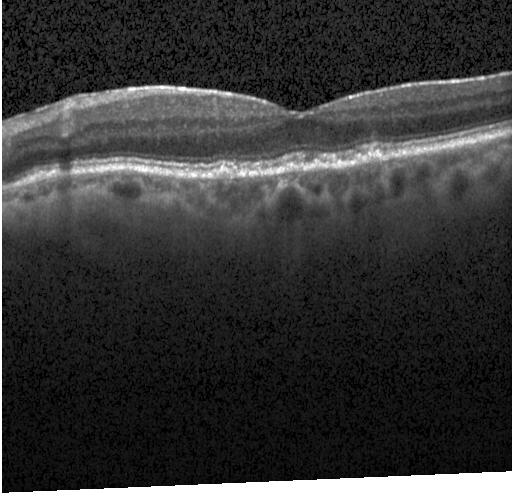

OCT B-scan showing multiple drusen.